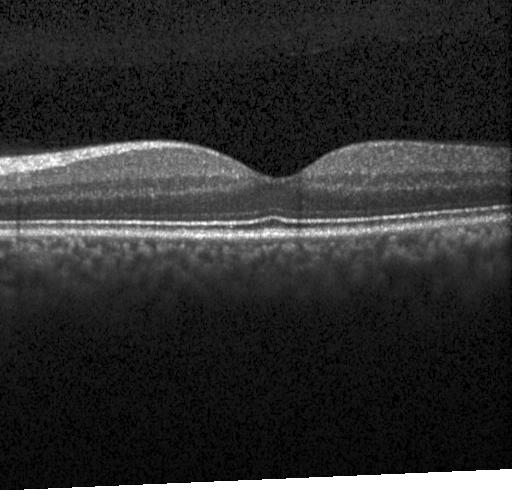 SD-OCT. OCT B-scan. Impression: neither CNV, DME, nor drusen.